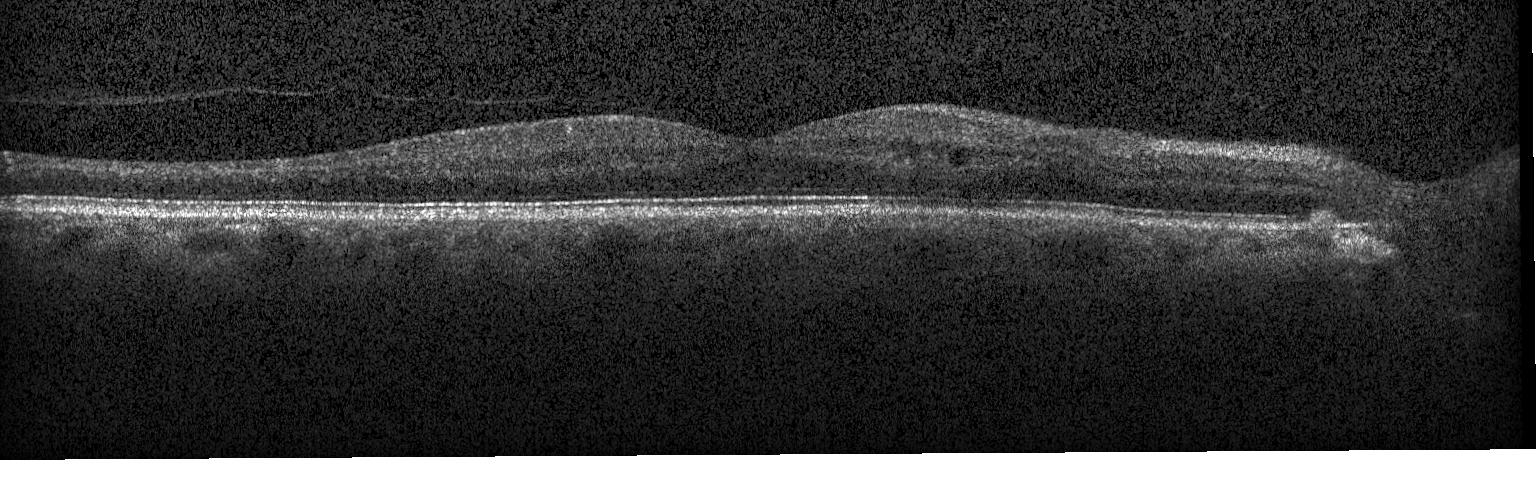
Retinal OCT cross-section showing diabetic macular edema (DME).